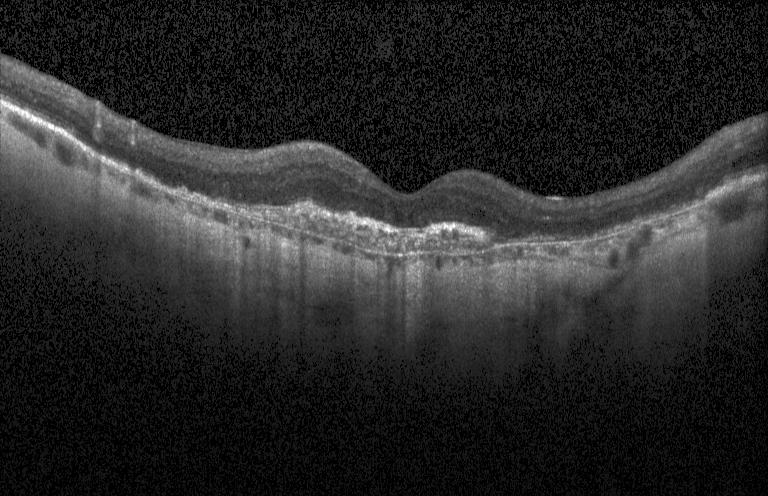 Choroidal neovascularization (CNV).